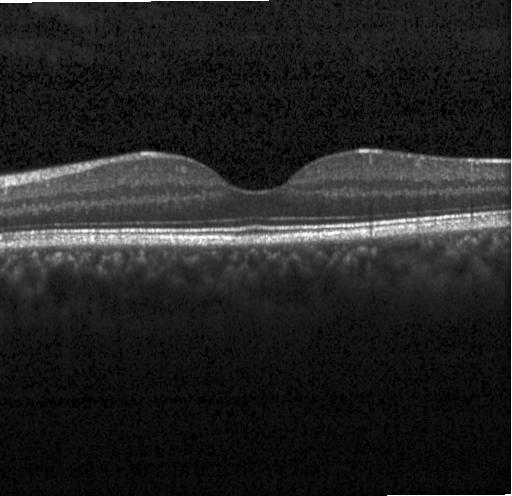
OCT line scan — Impression: neither choroidal neovascularization, diabetic macular edema, nor drusen.